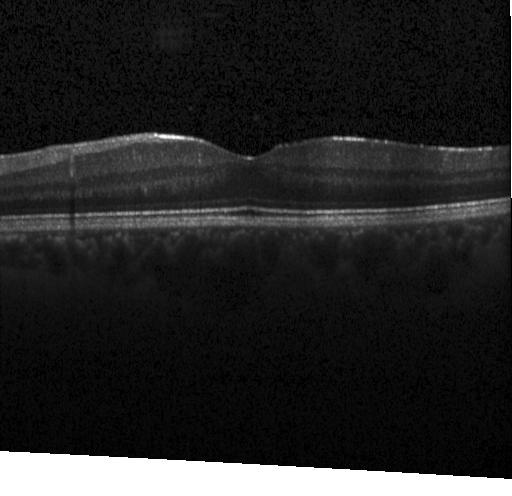 Retinal OCT cross-section, instrument: Heidelberg Spectralis, spectral-domain optical coherence tomography — Finding: neither choroidal neovascularization, diabetic macular edema, nor drusen.